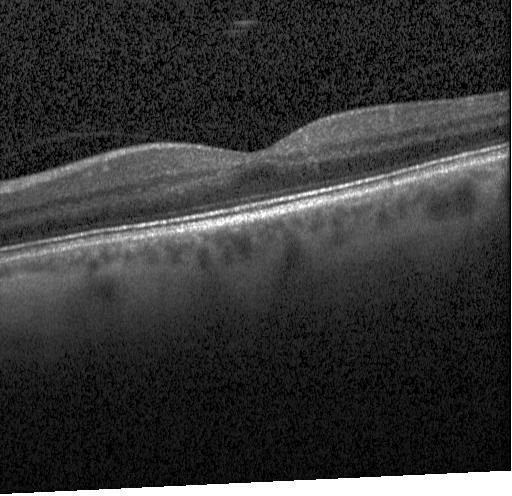 OCT B-scan; spectral-domain OCT; fovea-centered; Heidelberg Spectralis. This B-scan demonstrates neither CNV, DME, nor drusen.